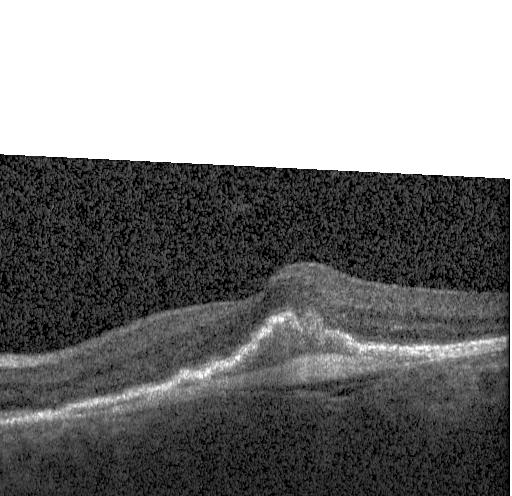 Optical coherence tomography scan, fovea-centered.
Diagnosis: a choroidal neovascular membrane.